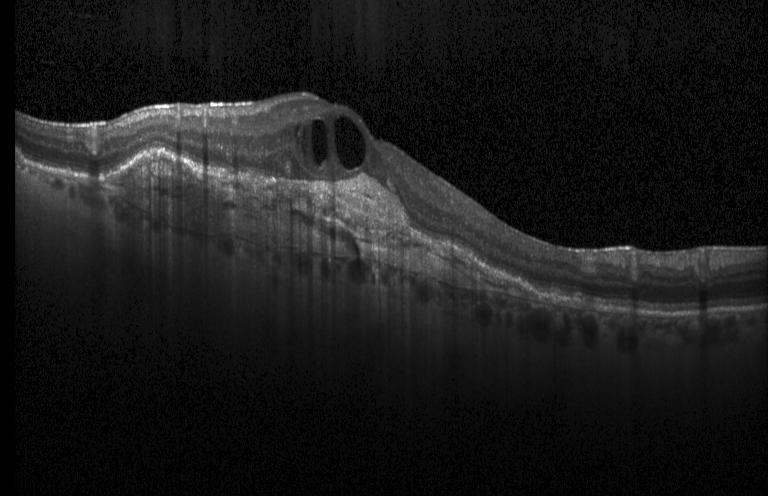

Spectral-domain OCT, retinal OCT B-scan, centered on the fovea, Heidelberg Spectralis.
Diagnosis: a choroidal neovascular membrane.